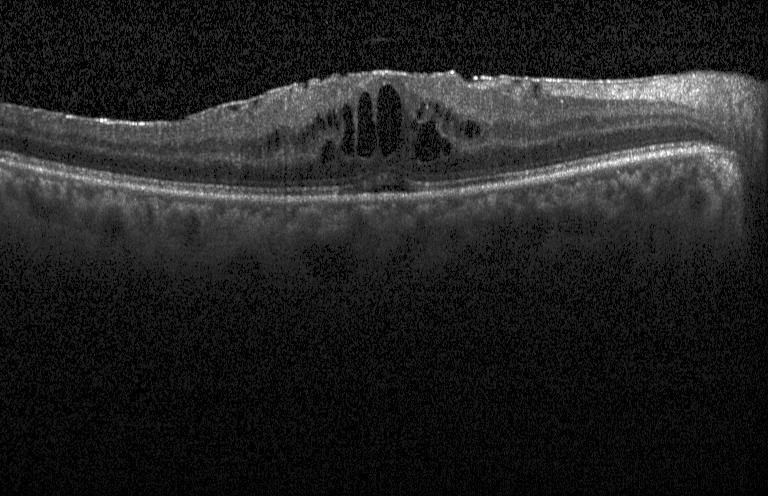

OCT line scan
Diagnosis: DME.